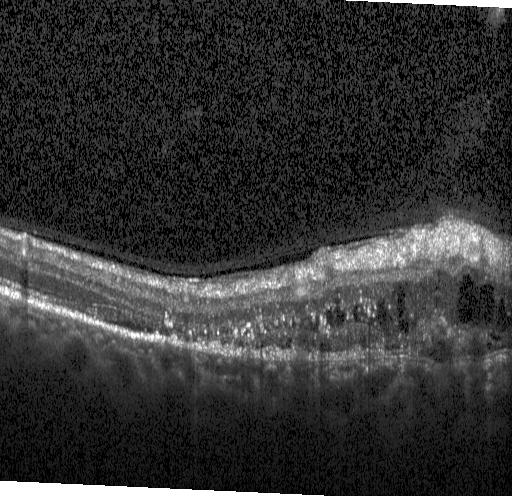

Finding: choroidal neovascularization (CNV).